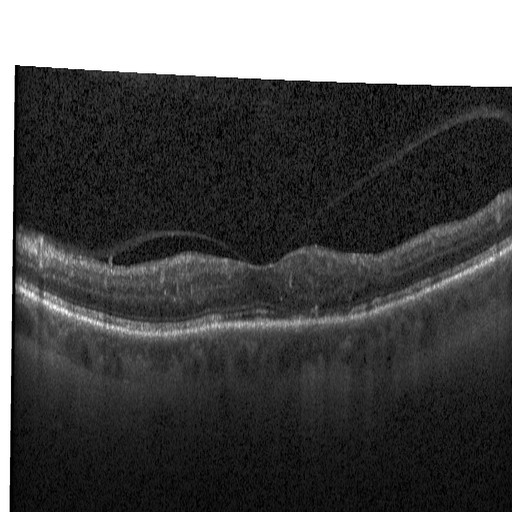 OCT B-scan showing diabetic macular edema (DME).